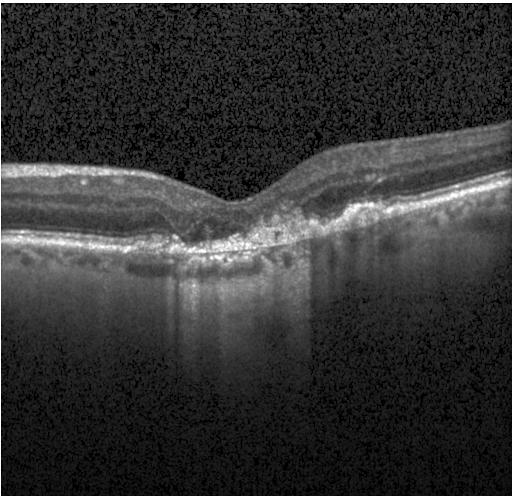

Heidelberg Spectralis OCT system; optical coherence tomography B-scan
Impression: a choroidal neovascular membrane.